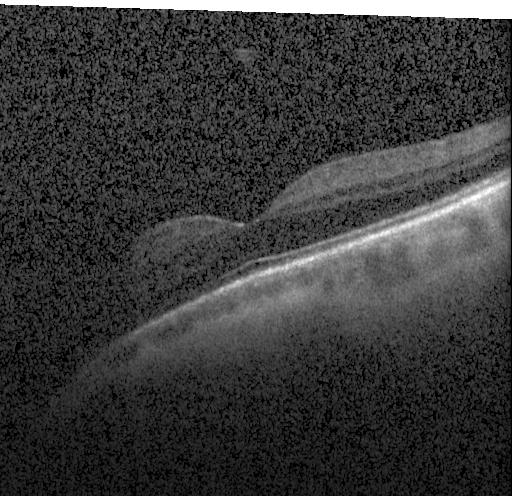
Dx: no choroidal neovascularization, no diabetic macular edema, and no drusen.